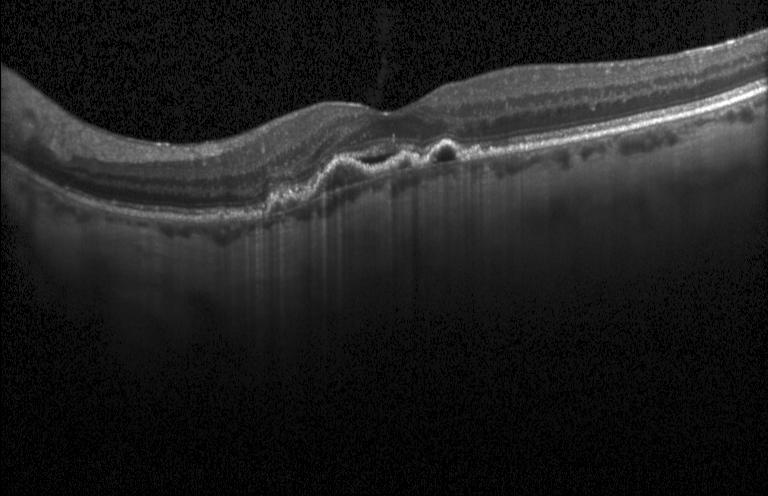 Optical coherence tomography B-scan · Heidelberg Spectralis OCT system · horizontal scan through the fovea. Finding: choroidal neovascularization.